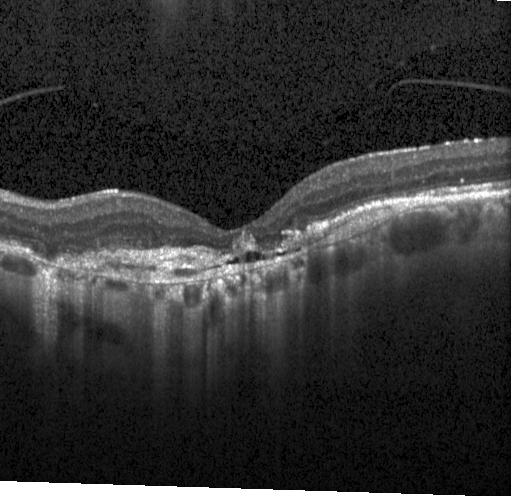 Through the macula · optical coherence tomography B-scan.
The scan shows a choroidal neovascular membrane.